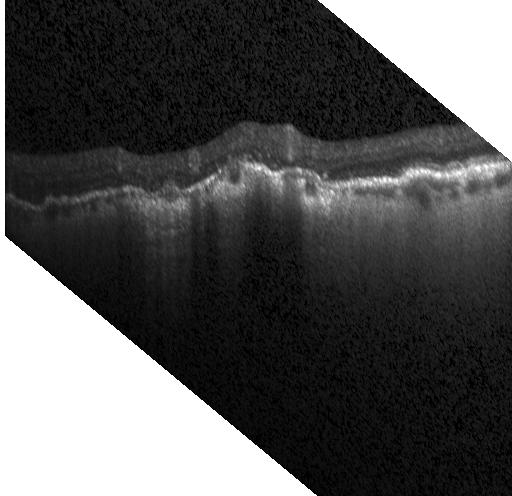
Choroidal neovascularization (CNV).